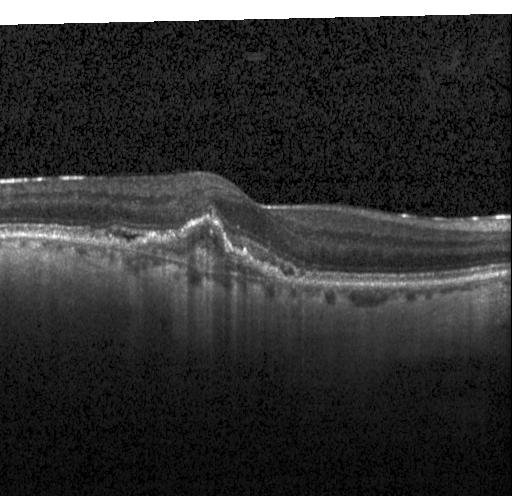
Impression: a choroidal neovascular membrane.